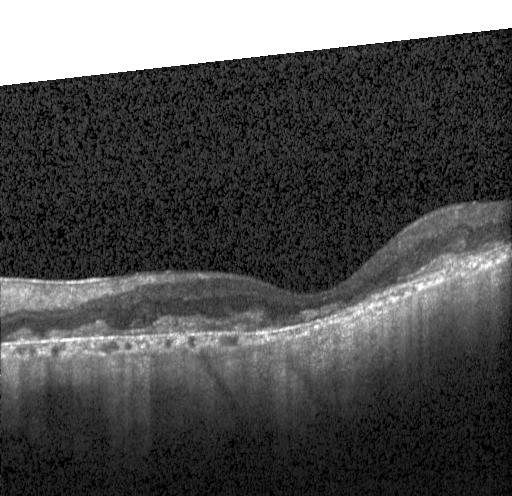

OCT line scan · spectral-domain OCT — Assessment: a choroidal neovascular membrane.